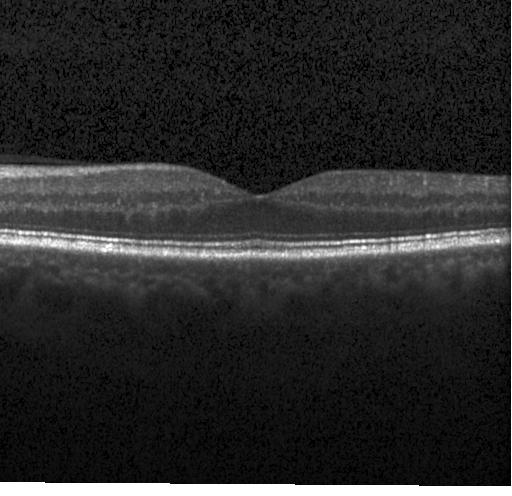
Heidelberg Spectralis. Through the macula. SD-OCT. Retinal OCT B-scan — This B-scan demonstrates neither choroidal neovascularization, diabetic macular edema, nor drusen.